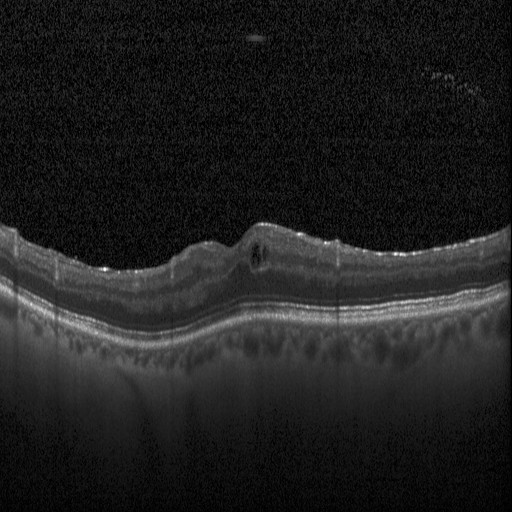

OCT B-scan, spectral-domain OCT, horizontal scan through the fovea, Heidelberg Spectralis — Impression: diabetic macular edema.